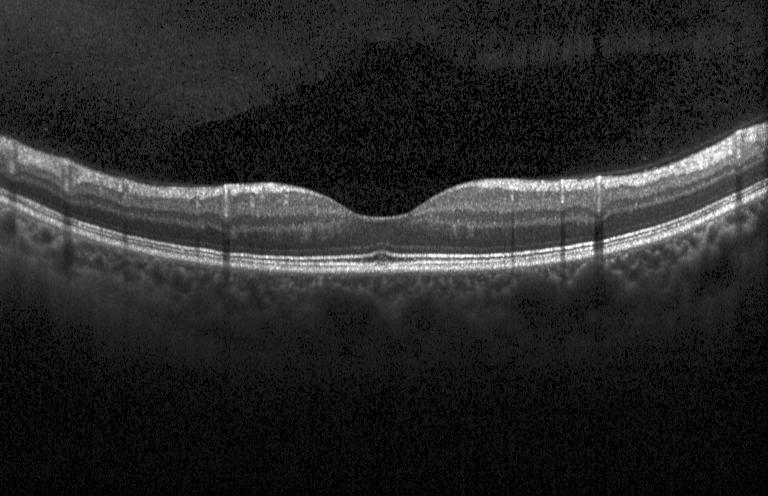 Diagnosis: no CNV, DME, or drusen.